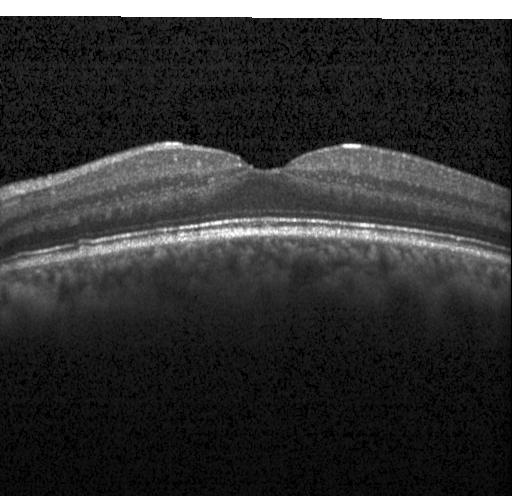

Acquired on a Heidelberg Spectralis, retinal OCT B-scan, through the macula — This B-scan demonstrates no evidence of CNV, DME, or drusen.